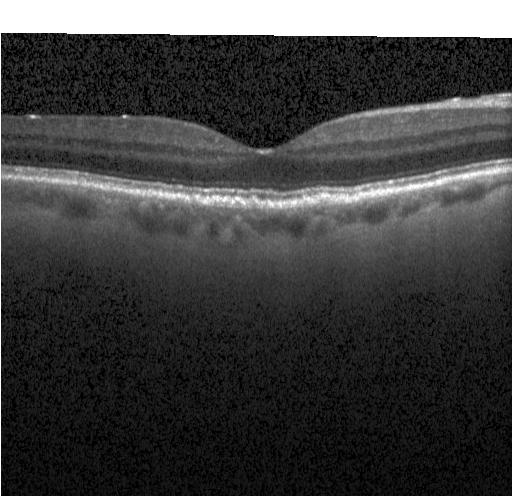

Optical coherence tomography scan. Macular scan. Impression: multiple drusen.